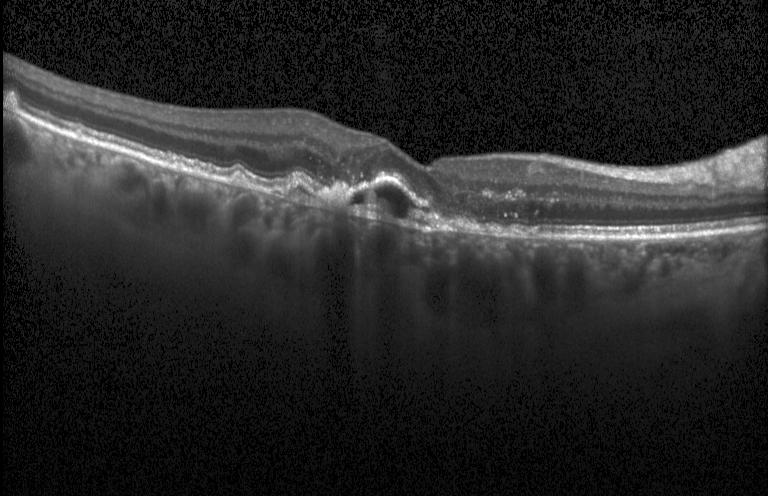 SD-OCT; OCT B-scan; Heidelberg Spectralis OCT system; macular scan — Impression: a choroidal neovascular membrane.